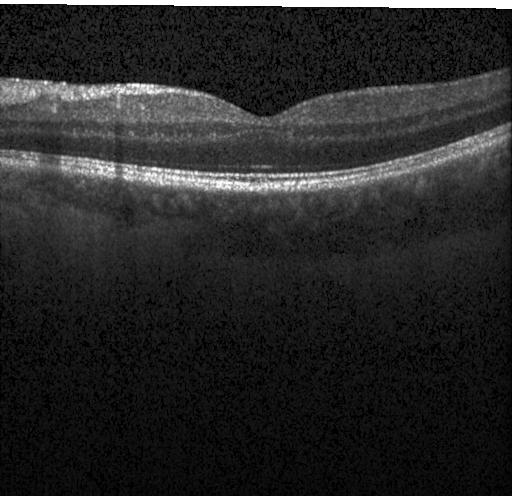

Optical coherence tomography scan. Centered on the fovea. Acquired on a Heidelberg Spectralis. SD-OCT — Diagnosis: neither CNV, DME, nor drusen.